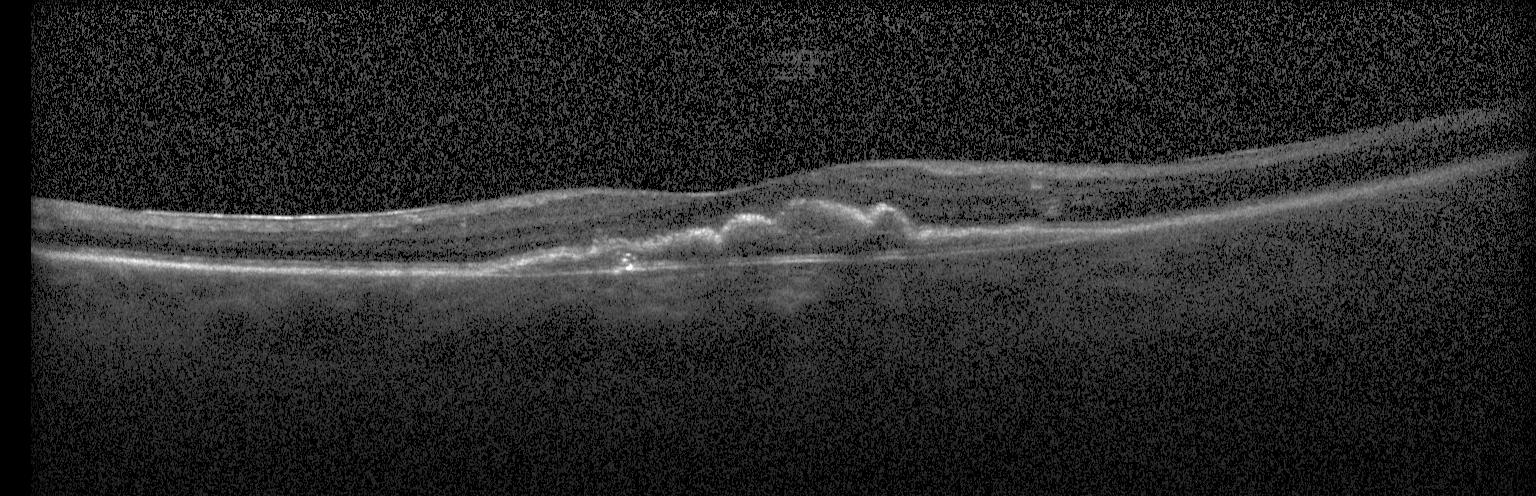 Through the macula; retinal OCT B-scan; instrument: Heidelberg Spectralis; spectral-domain optical coherence tomography. The scan shows choroidal neovascularization.